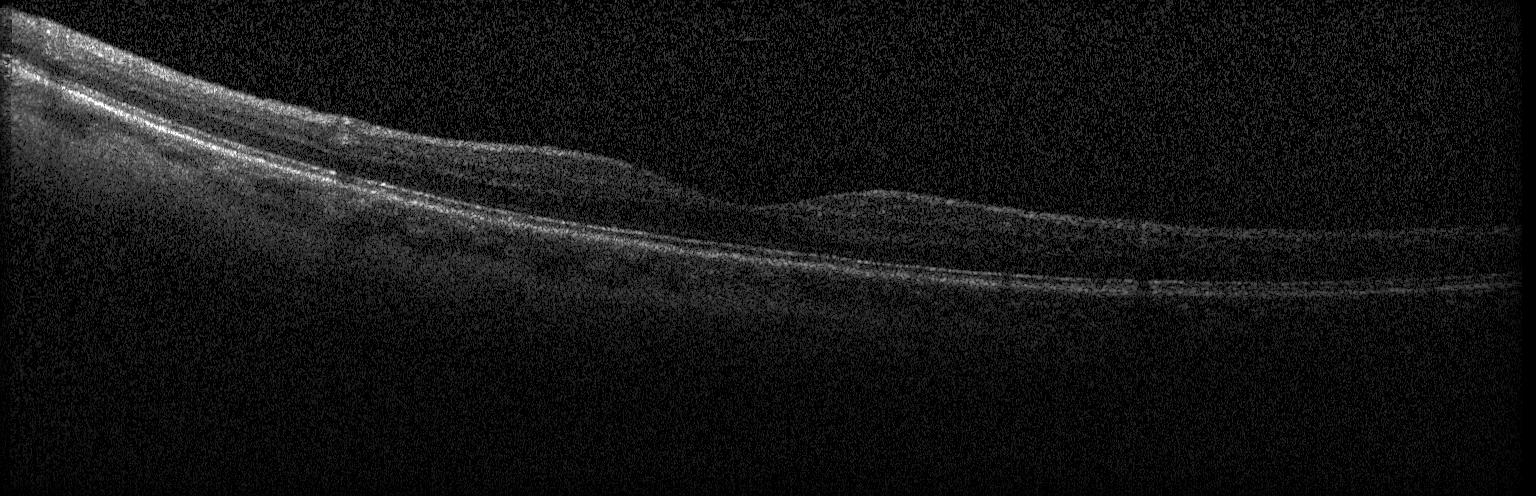
Diagnosis: no CNV, DME, or drusen.